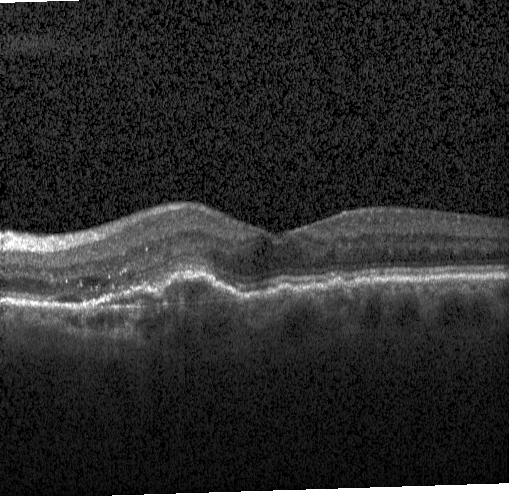

OCT scan showing CNV.